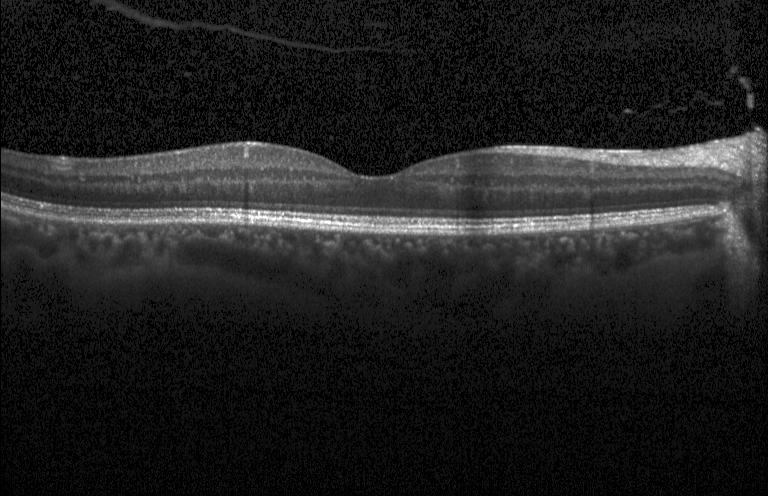

Retinal OCT B-scan, spectral-domain optical coherence tomography, macular scan, Heidelberg Spectralis — Finding: neither choroidal neovascularization, diabetic macular edema, nor drusen.